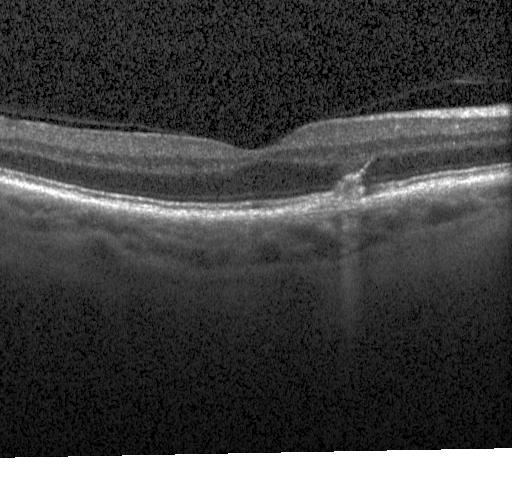

Dx: drusen.